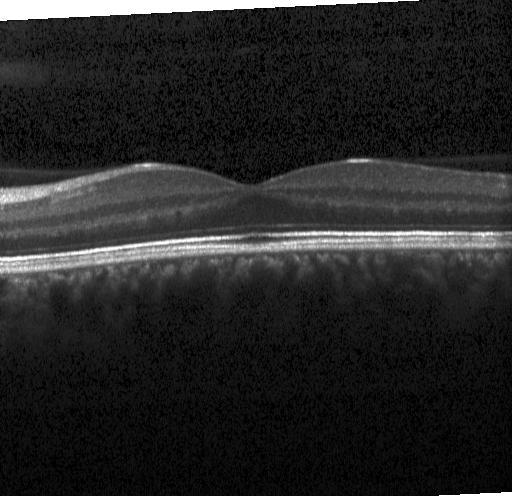

Impression: no evidence of CNV, DME, or drusen.